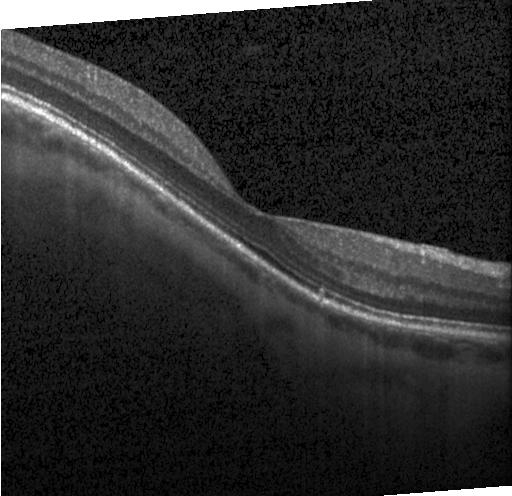
Finding: no choroidal neovascularization, diabetic macular edema, or drusen.